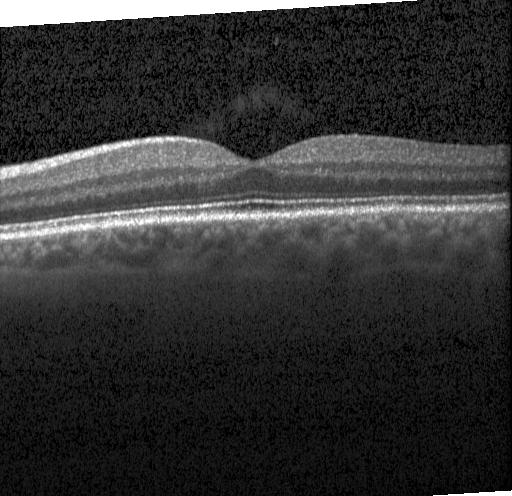 Retinal OCT cross-section · fovea-centered · spectral-domain optical coherence tomography · Heidelberg Spectralis. Diagnosis: neither choroidal neovascularization, diabetic macular edema, nor drusen.